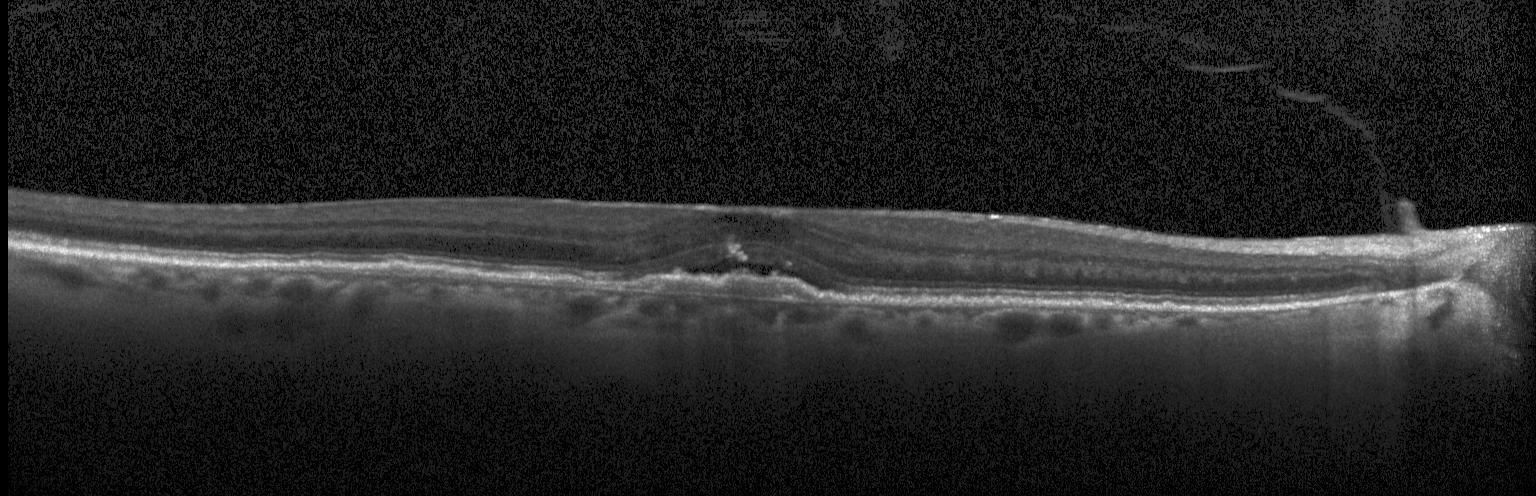
Optical coherence tomography scan. SD-OCT. This B-scan demonstrates a choroidal neovascular membrane.